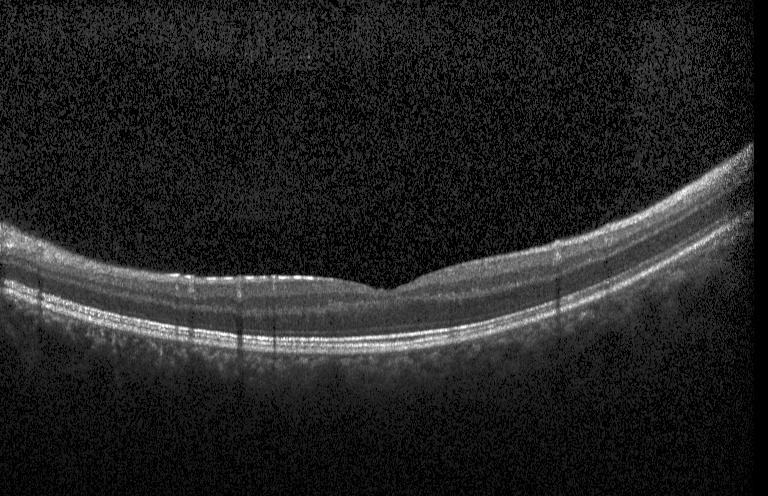

Finding: no evidence of choroidal neovascularization, diabetic macular edema, or drusen.